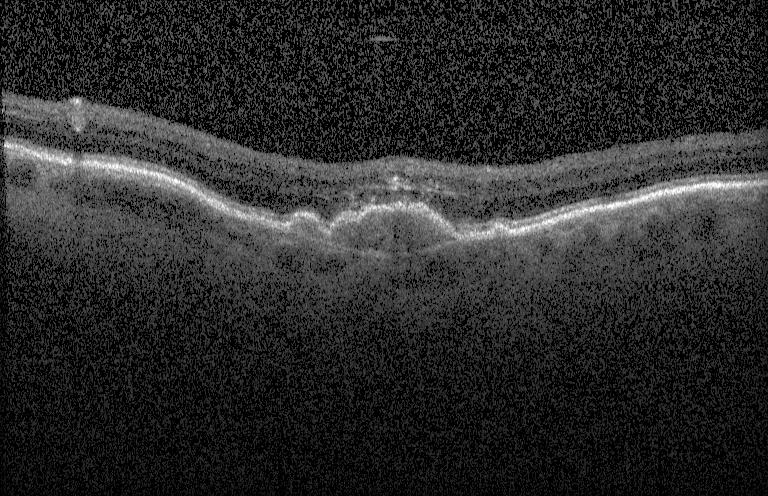
Macular scan. SD-OCT. Optical coherence tomography B-scan — Finding: a choroidal neovascular membrane.